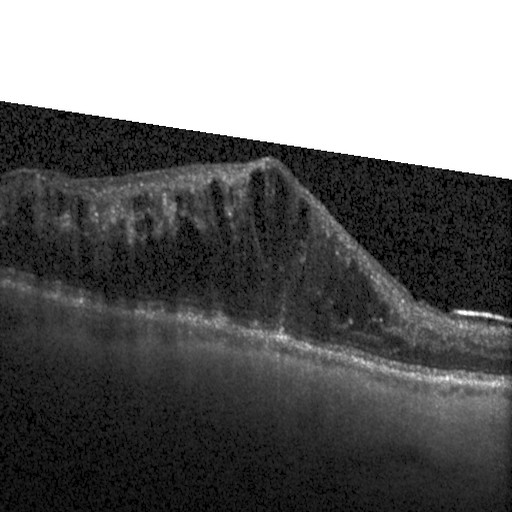

OCT line scan — OCT finding: diabetic macular edema (DME).